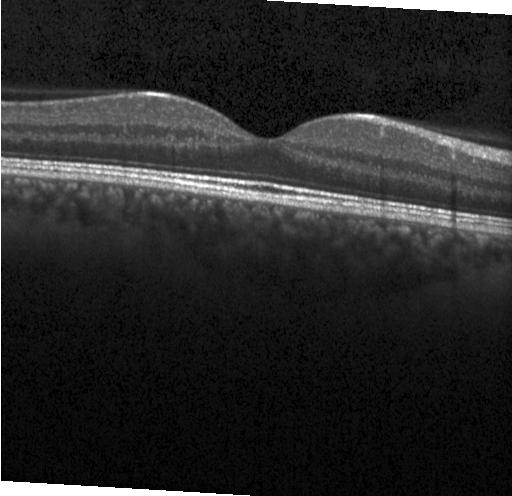
Centered on the fovea · optical coherence tomography scan.
Diagnosis: neither choroidal neovascularization, diabetic macular edema, nor drusen.